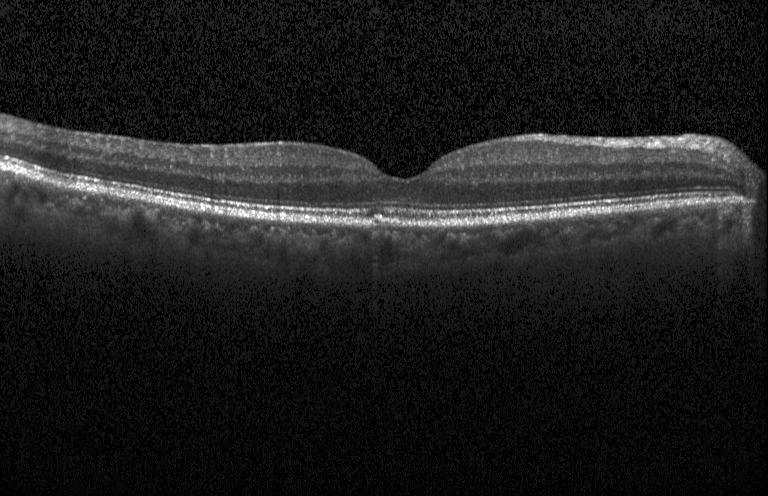

Optical coherence tomography scan; horizontal scan through the fovea.
No CNV, DME, or drusen.